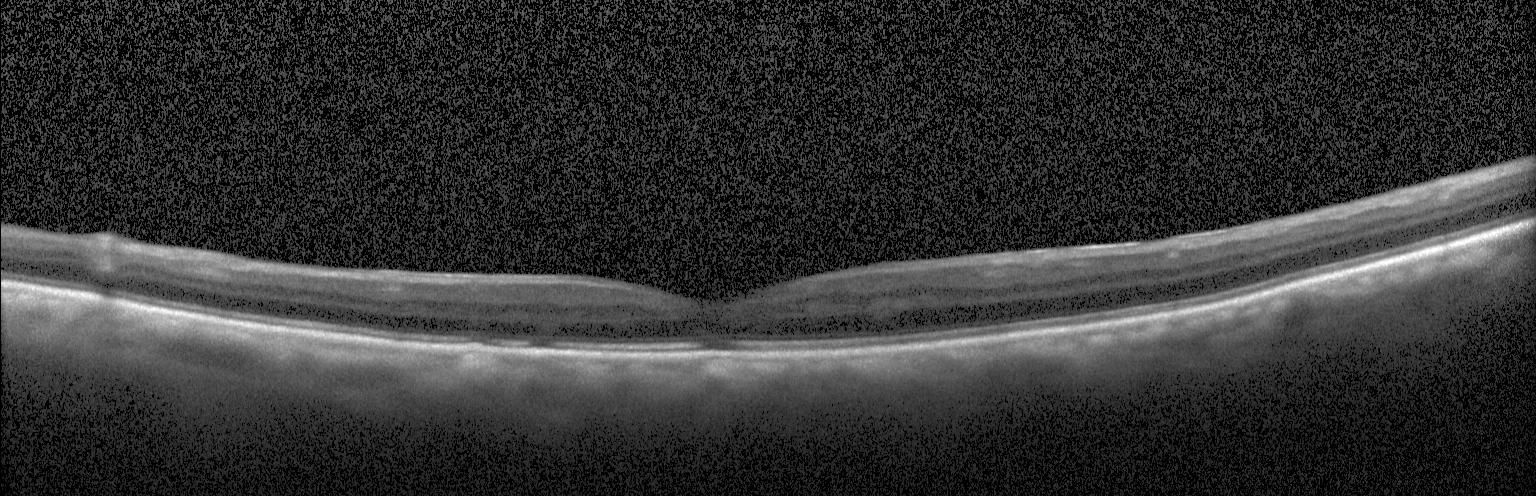

OCT scan showing no choroidal neovascularization, no diabetic macular edema, and no drusen.